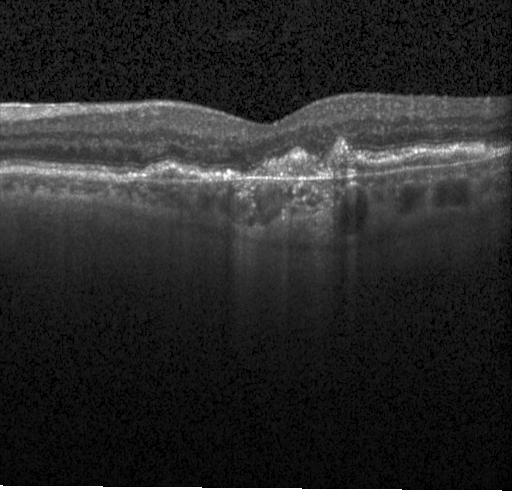 Macular OCT demonstrating choroidal neovascularization (CNV).